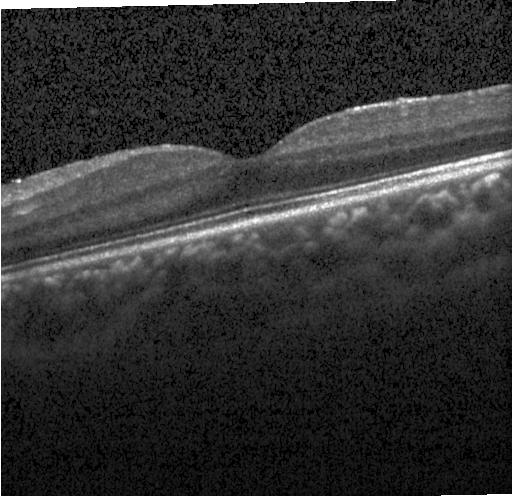 Optical coherence tomography scan. Finding: no evidence of choroidal neovascularization, diabetic macular edema, or drusen.